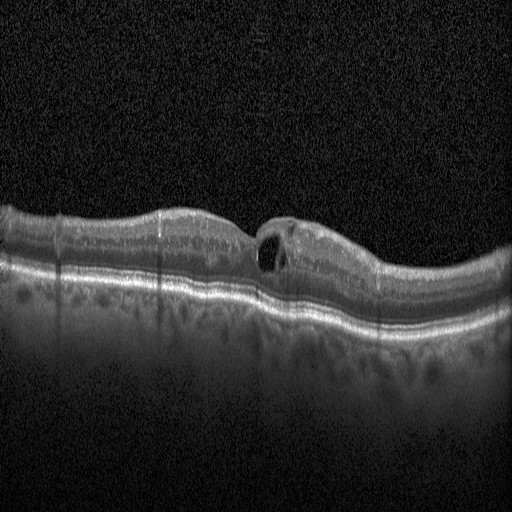 Macular scan · spectral-domain OCT · Heidelberg Spectralis OCT system · retinal OCT B-scan. Assessment: diabetic macular edema (DME).